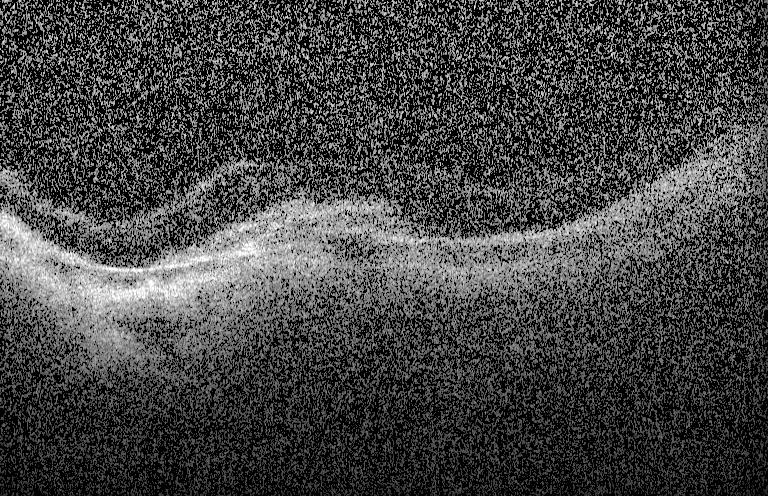 Macular OCT: a choroidal neovascular membrane.